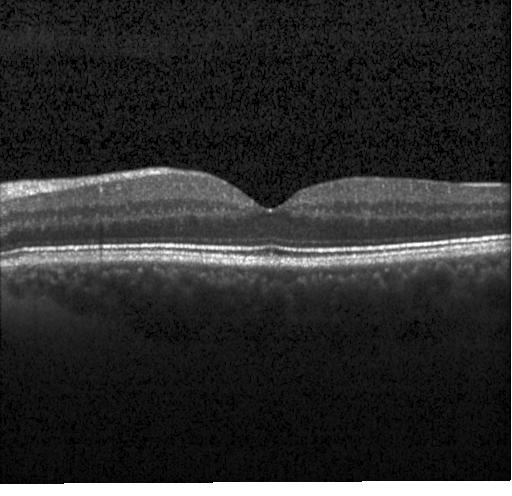 OCT line scan; spectral-domain OCT. Impression: no evidence of CNV, DME, or drusen.